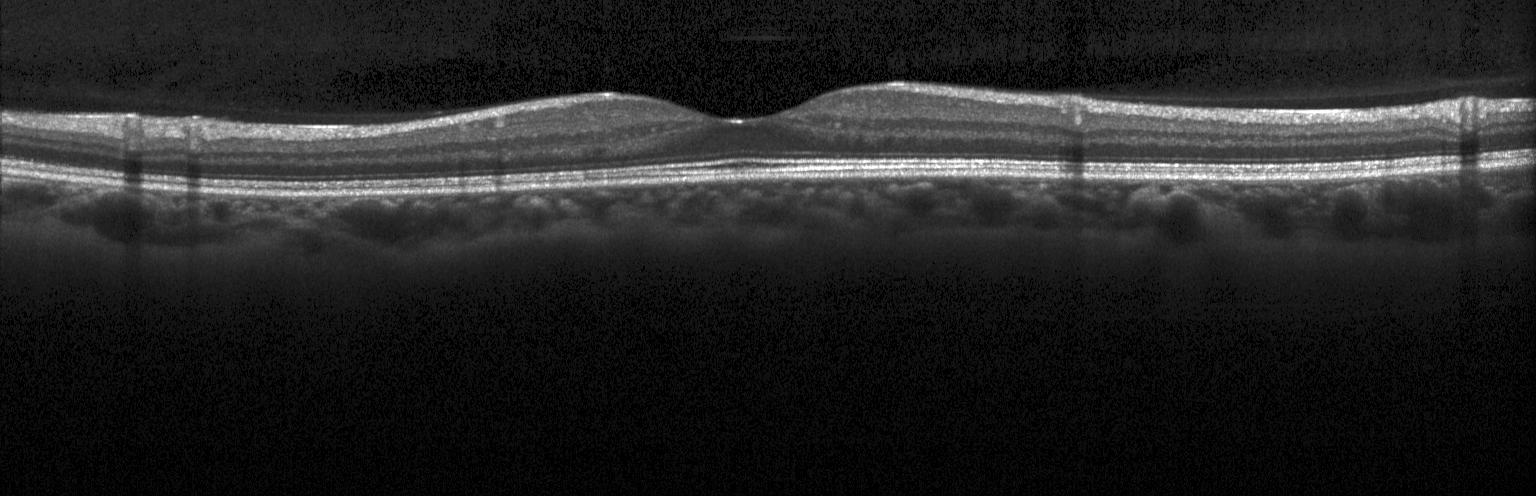
Finding: no CNV, no DME, and no drusen.